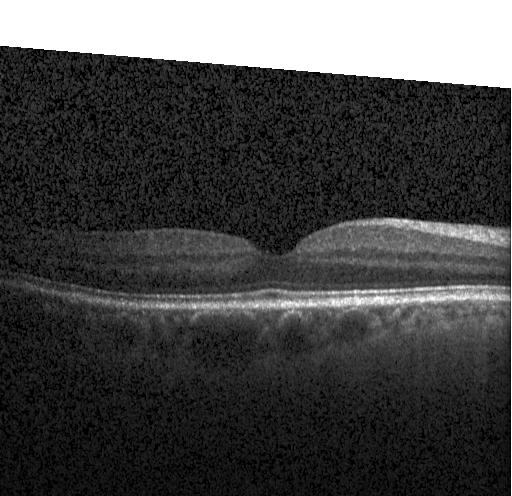 OCT line scan. Heidelberg Spectralis OCT system — Diagnosis: neither choroidal neovascularization, diabetic macular edema, nor drusen.